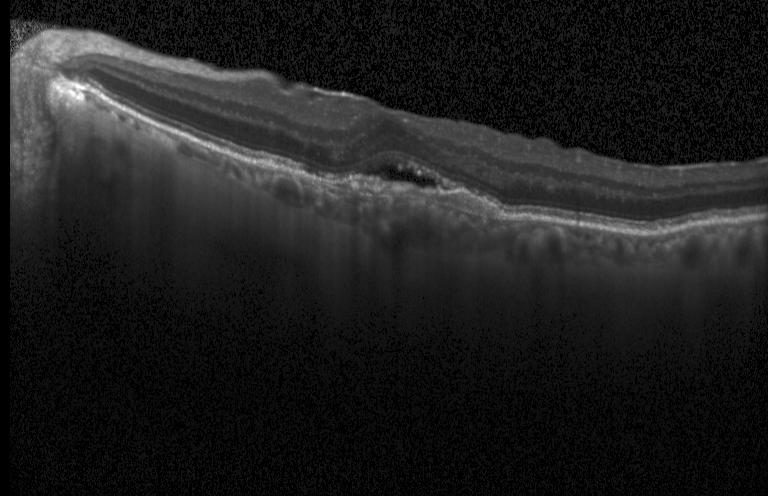 Macular OCT demonstrating choroidal neovascularization.